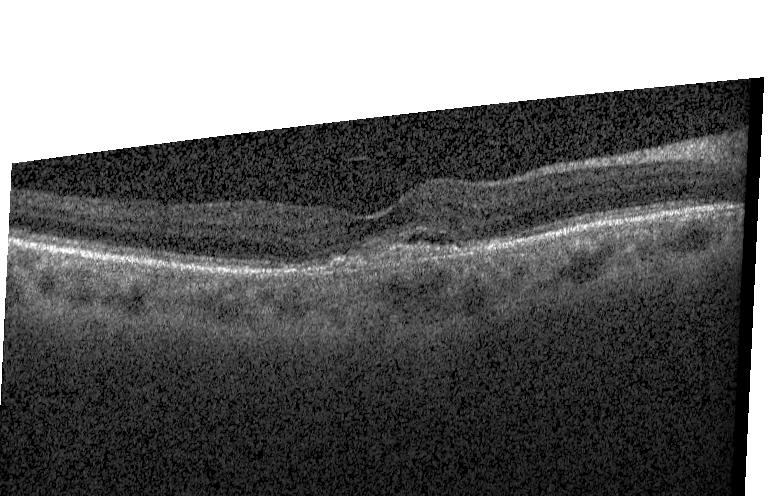
Fovea-centered. Instrument: Heidelberg Spectralis. Optical coherence tomography B-scan. Impression: choroidal neovascularization (CNV).